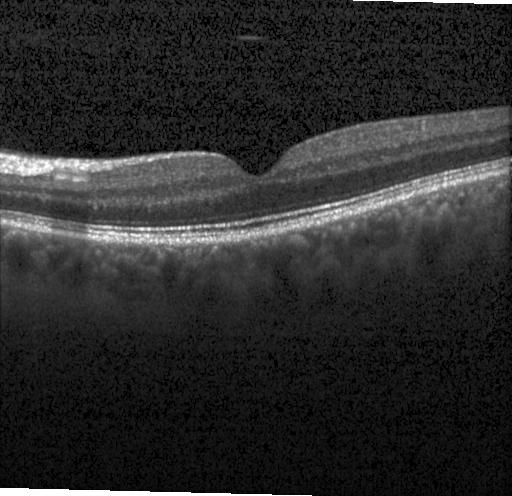 OCT B-scan showing no choroidal neovascularization, no diabetic macular edema, and no drusen.